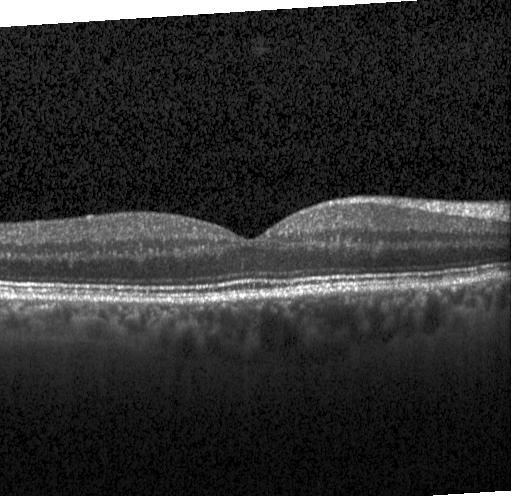 Spectral-domain OCT; optical coherence tomography B-scan; Heidelberg Spectralis OCT system.
Impression: no evidence of choroidal neovascularization, diabetic macular edema, or drusen.